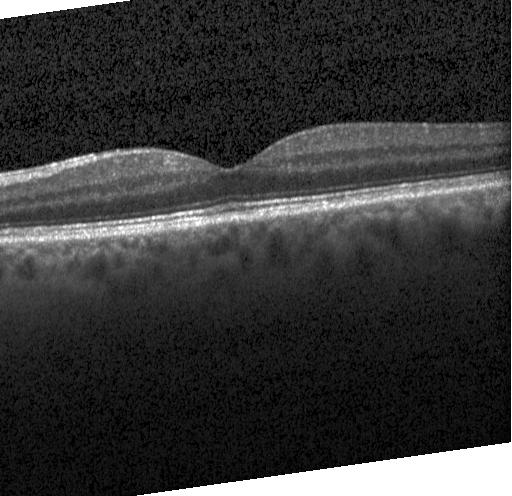

OCT B-scan
Diagnosis: no evidence of choroidal neovascularization, diabetic macular edema, or drusen.